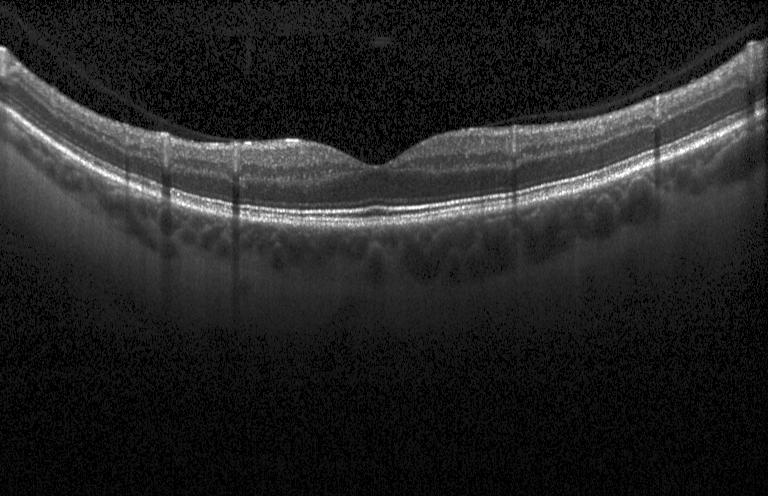
Dx: no choroidal neovascularization, no diabetic macular edema, and no drusen.